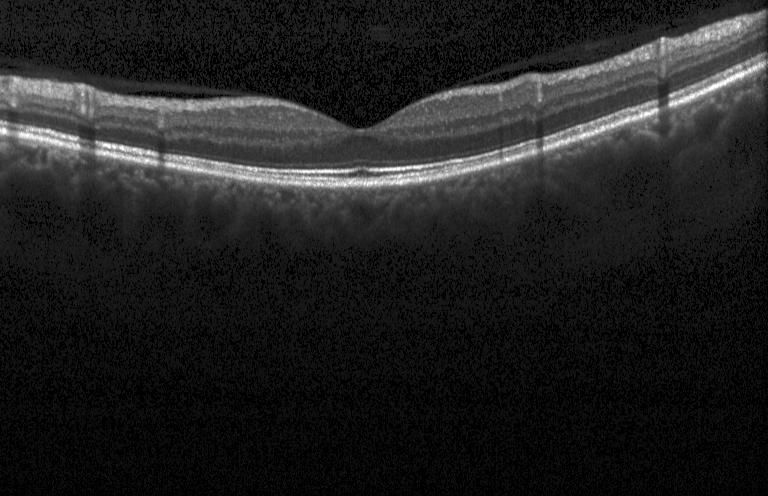

Diagnosis: neither choroidal neovascularization, diabetic macular edema, nor drusen.